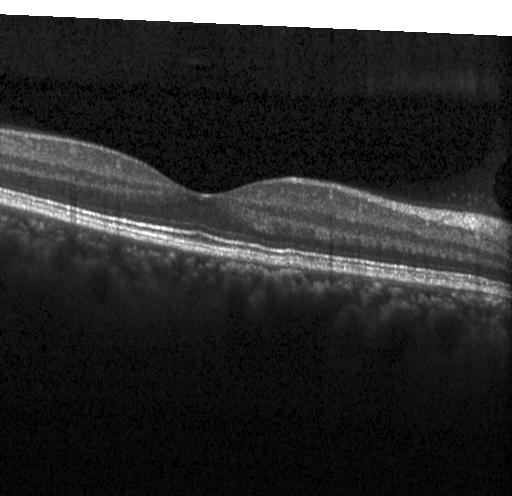
Through the macula · retinal OCT B-scan. Finding: no choroidal neovascularization, diabetic macular edema, or drusen.